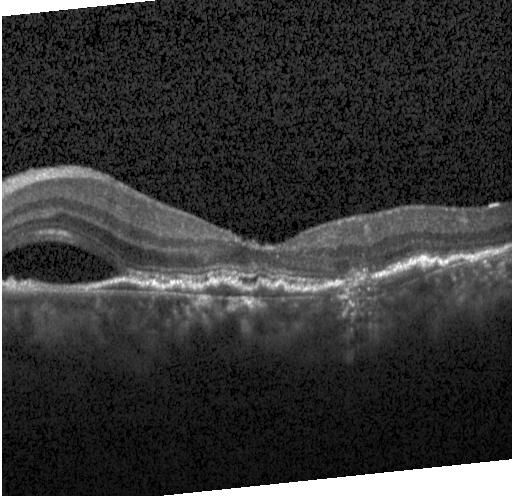

OCT B-scan. A choroidal neovascular membrane.